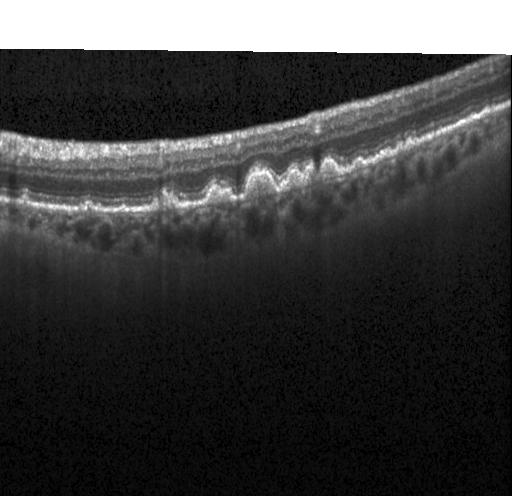

The scan shows drusen.